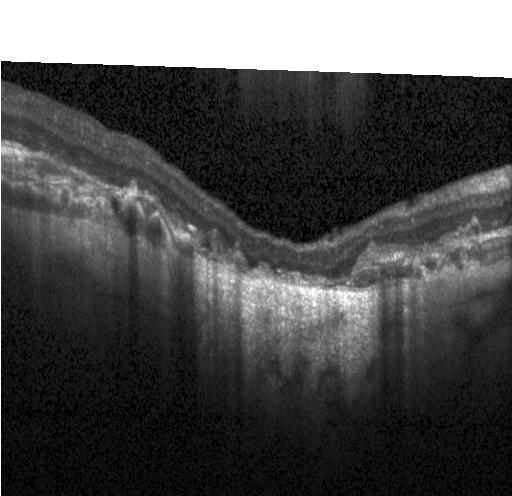

Spectral-domain OCT, Heidelberg Spectralis, through the macula, retinal OCT cross-section
Impression: choroidal neovascularization (CNV).